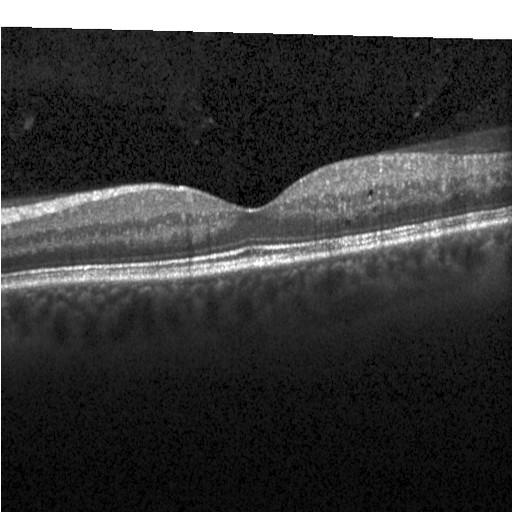

SD-OCT; acquired on a Heidelberg Spectralis; OCT B-scan; centered on the fovea. Finding: diabetic macular edema (DME).